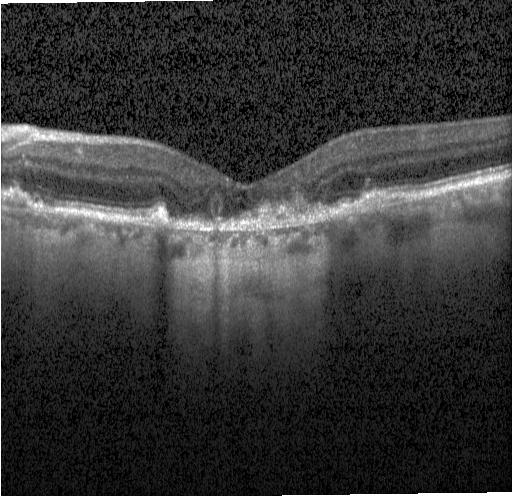
OCT scan showing a choroidal neovascular membrane.